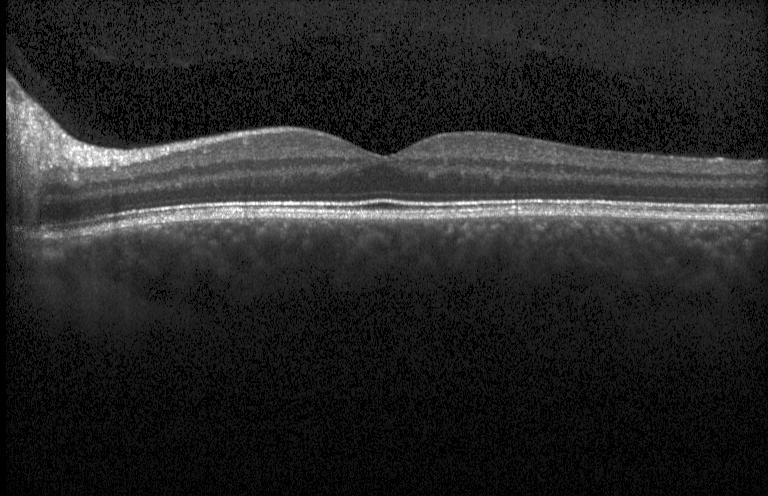 Centered on the fovea; spectral-domain OCT; acquired on a Heidelberg Spectralis; optical coherence tomography B-scan — Diagnosis: no evidence of choroidal neovascularization, diabetic macular edema, or drusen.